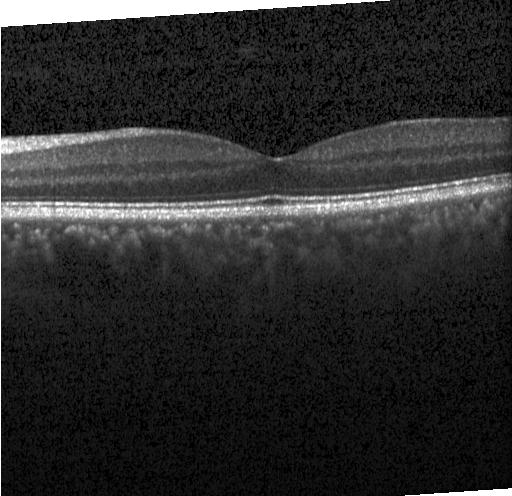
Retinal OCT cross-section, centered on the fovea
Diagnosis: neither choroidal neovascularization, diabetic macular edema, nor drusen.